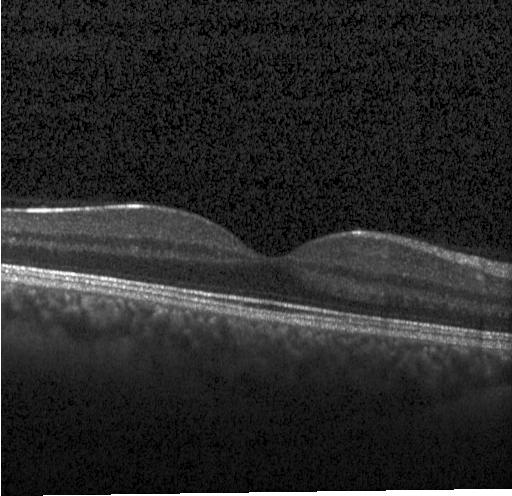

Optical coherence tomography B-scan.
OCT finding: no choroidal neovascularization, no diabetic macular edema, and no drusen.